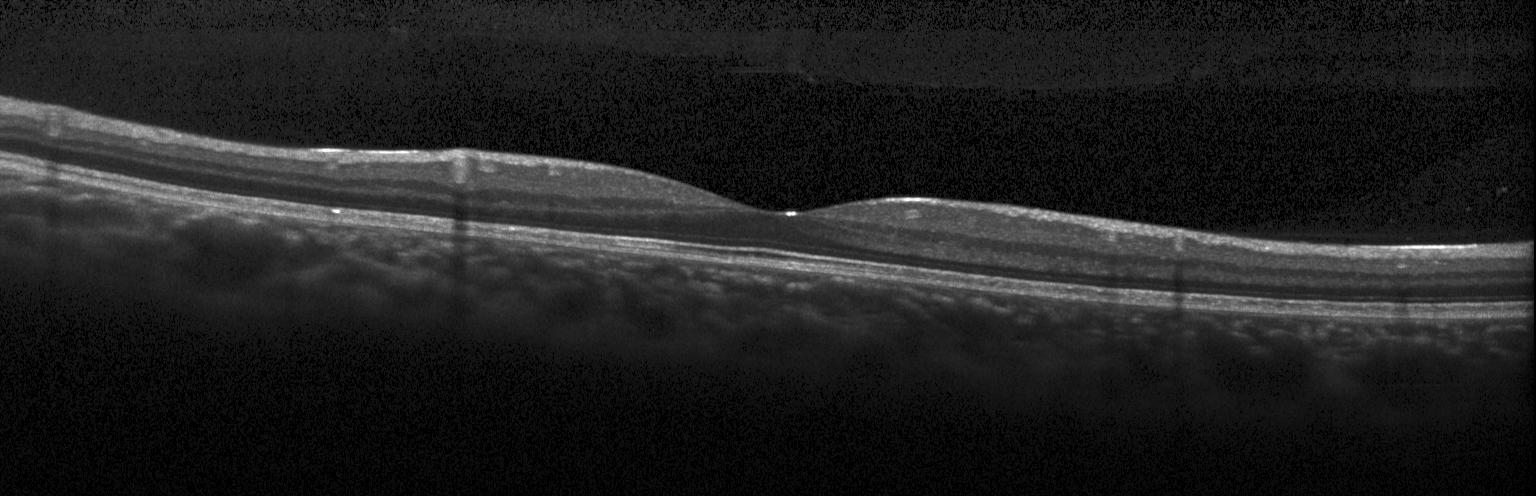
Macular OCT: no CNV, no DME, and no drusen.